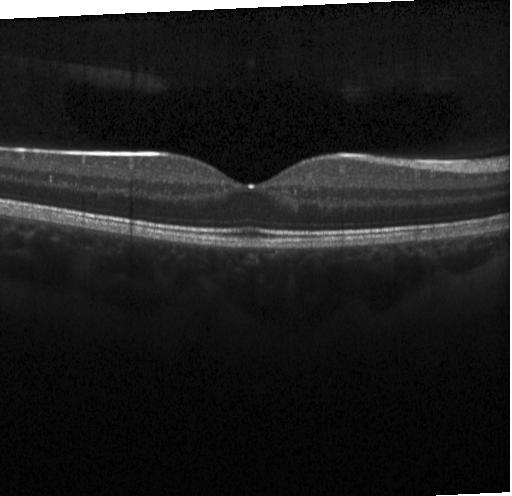
Diagnosis: no CNV, DME, or drusen.